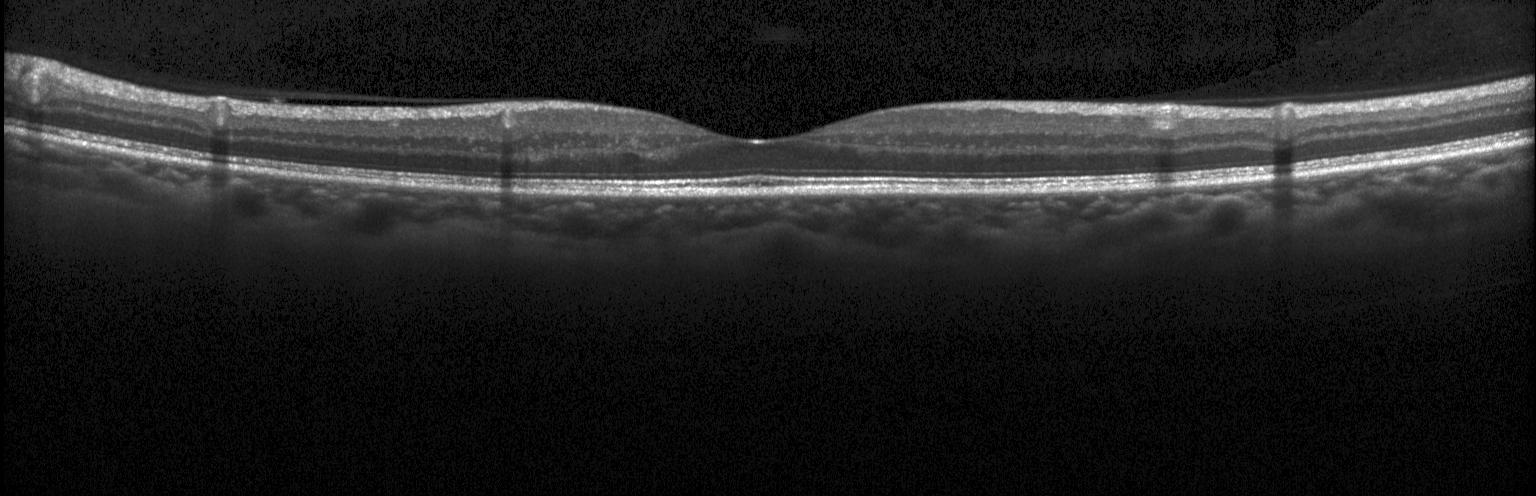 Retinal OCT B-scan — OCT finding: no choroidal neovascularization, diabetic macular edema, or drusen.